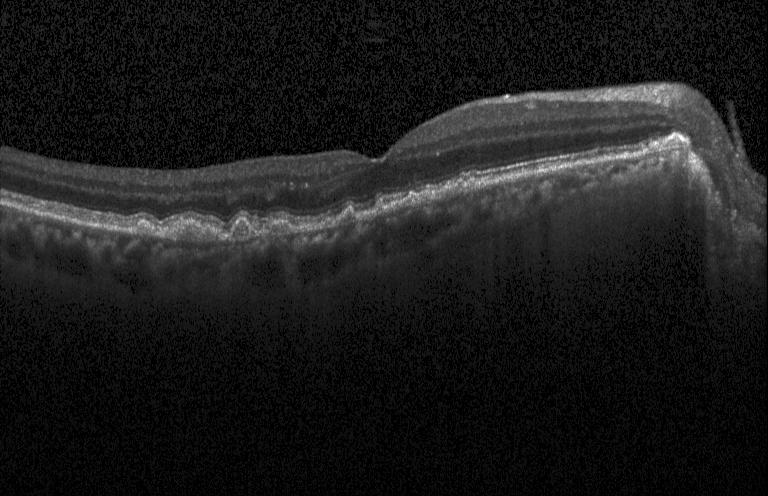
Retinal OCT cross-section; instrument: Heidelberg Spectralis — The scan shows multiple drusen.